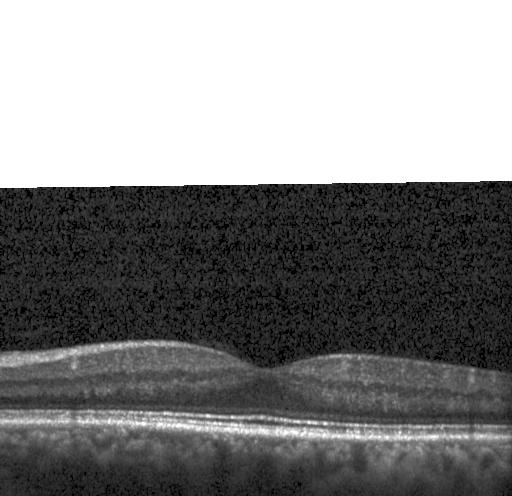

Assessment: neither CNV, DME, nor drusen.